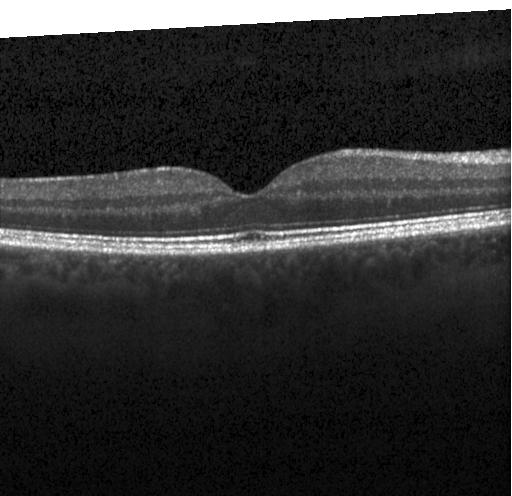 Diagnosis: no choroidal neovascularization, no diabetic macular edema, and no drusen.